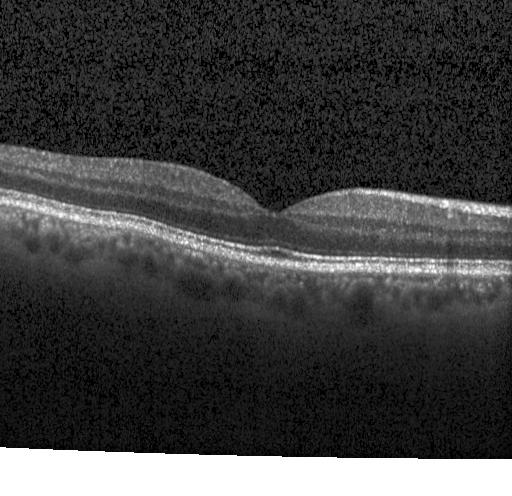
Dx: no CNV, no DME, and no drusen.